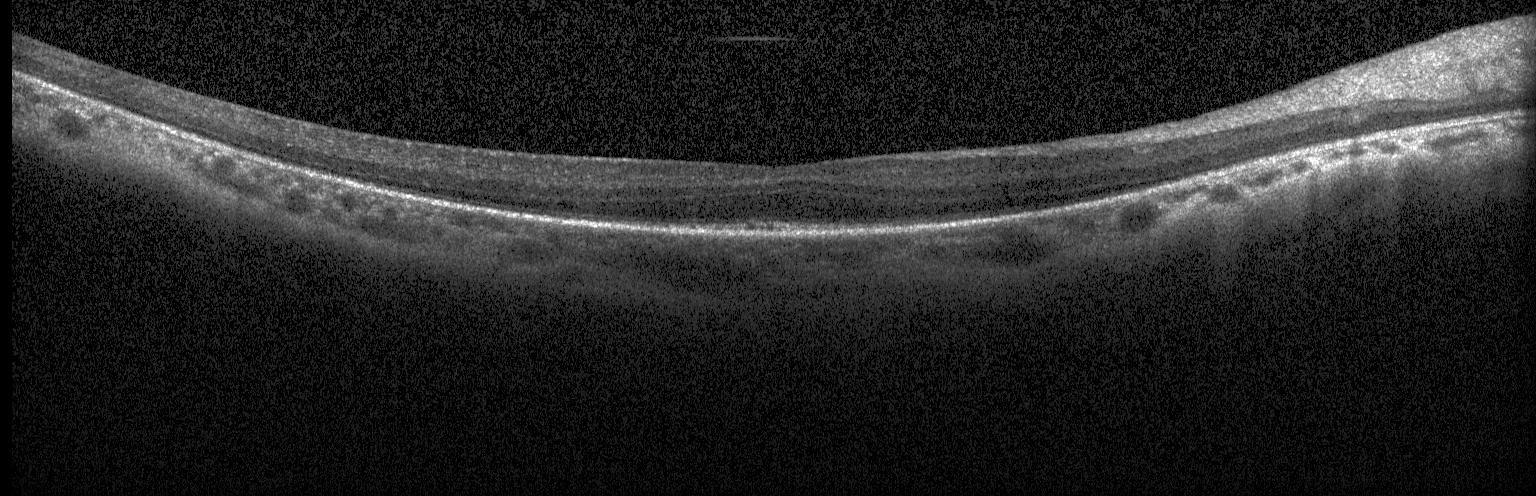 Retinal OCT cross-section showing no choroidal neovascularization, diabetic macular edema, or drusen.